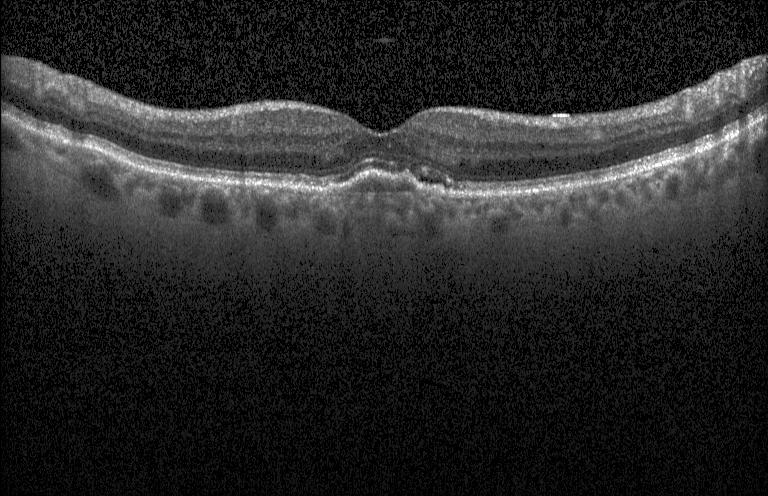 Retinal OCT cross-section showing a choroidal neovascular membrane.